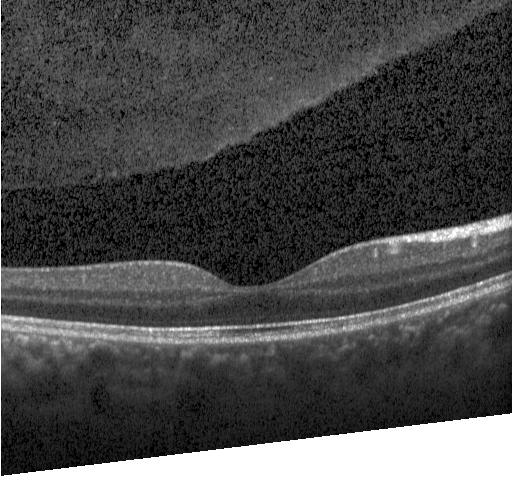
OCT B-scan; Heidelberg Spectralis OCT system.
Assessment: no evidence of CNV, DME, or drusen.